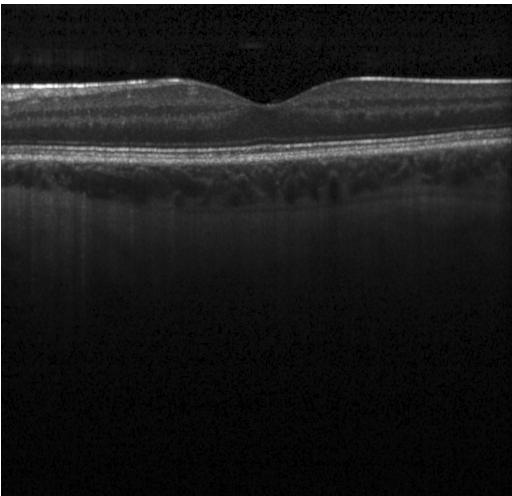
Horizontal scan through the fovea. Spectral-domain OCT. OCT line scan
Assessment: neither CNV, DME, nor drusen.